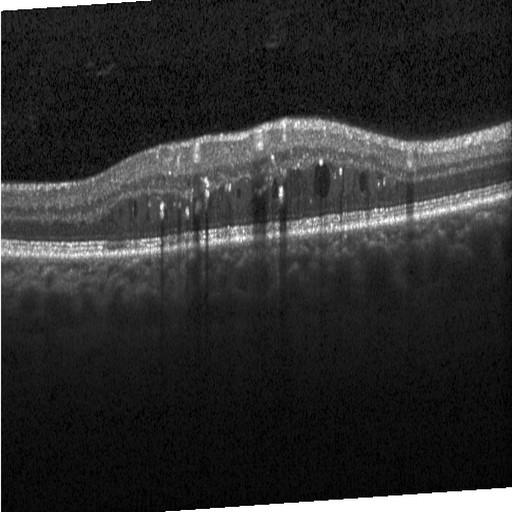

OCT line scan; centered on the fovea. Finding: diabetic macular edema.